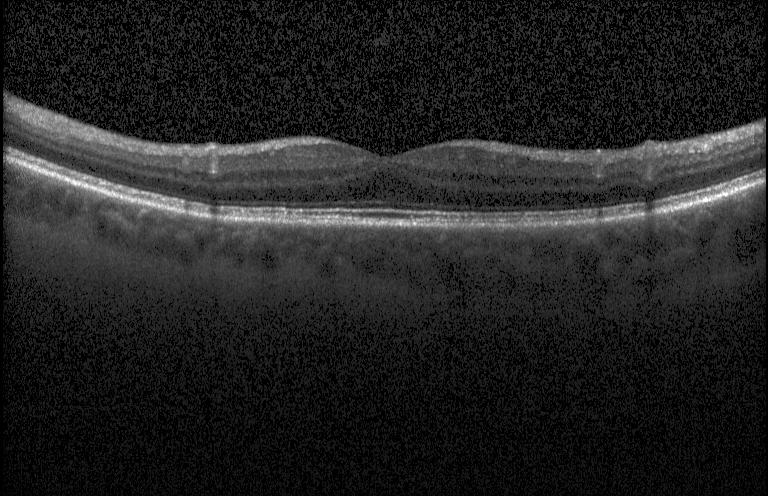

Optical coherence tomography B-scan, instrument: Heidelberg Spectralis, SD-OCT.
Macular OCT: no CNV, no DME, and no drusen.